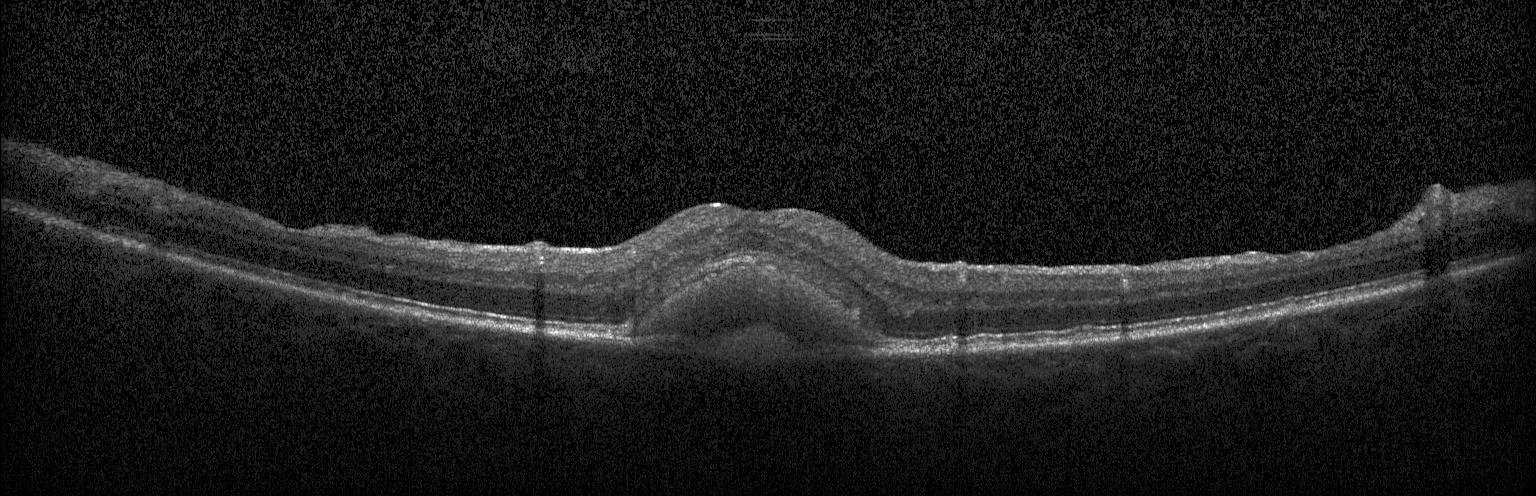
Spectral-domain OCT. Retinal OCT cross-section. Heidelberg Spectralis. Macular scan
Finding: choroidal neovascularization (CNV).